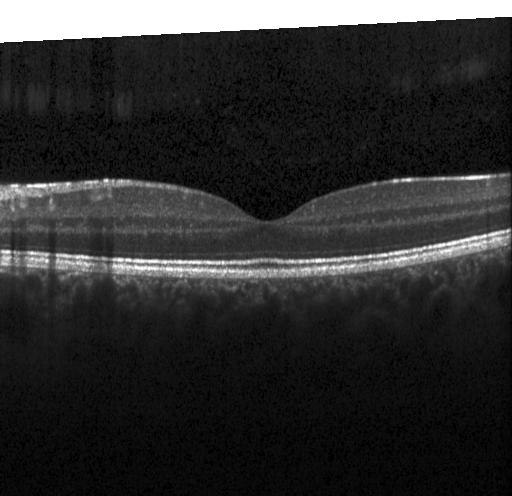 Retinal OCT B-scan, centered on the fovea, SD-OCT — Macular OCT: no evidence of choroidal neovascularization, diabetic macular edema, or drusen.